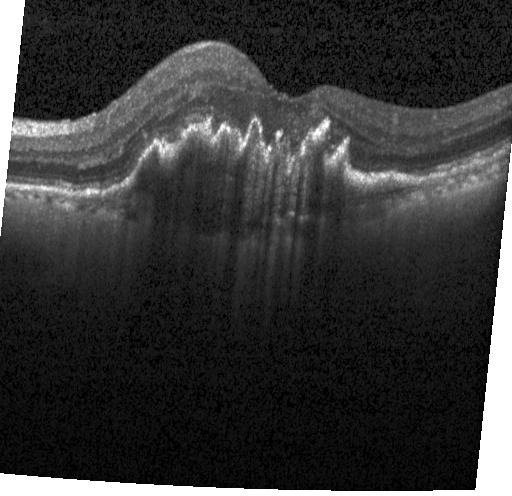

Centered on the fovea. Heidelberg Spectralis OCT system. OCT line scan
Macular OCT: CNV.